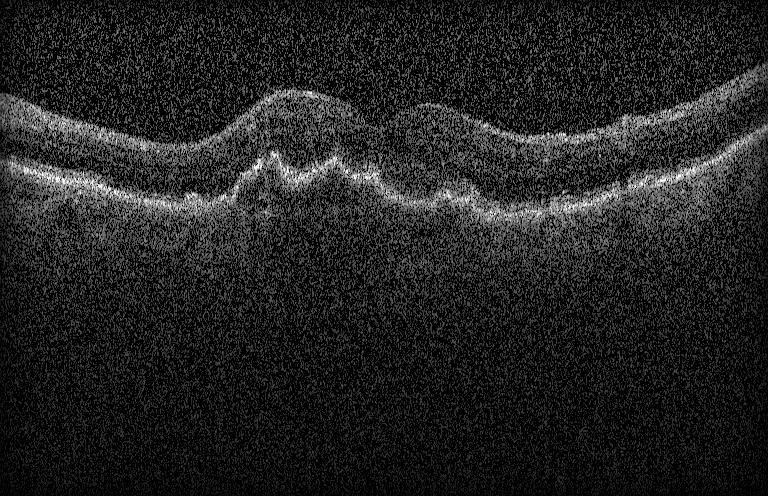
OCT scan showing CNV.